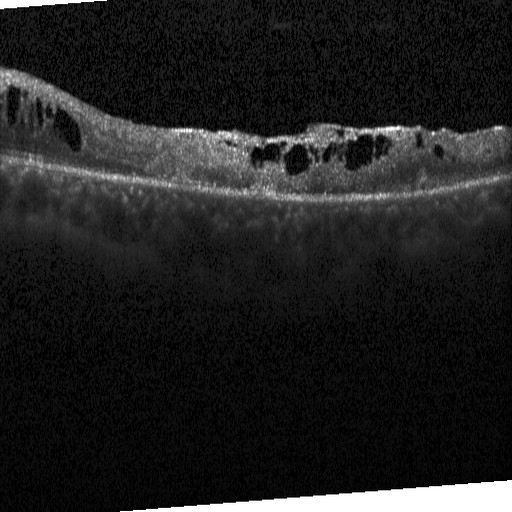 Finding: diabetic macular edema (DME).